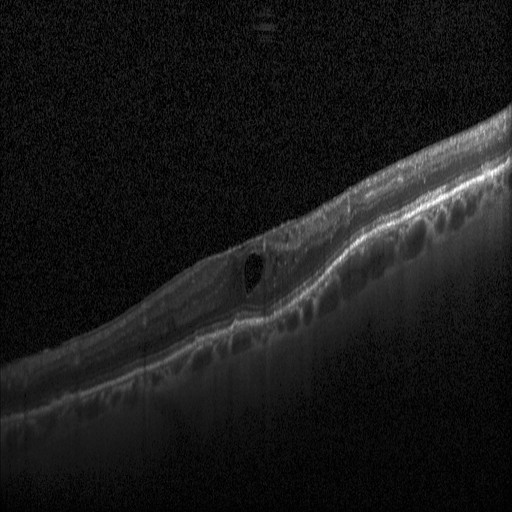

Assessment: DME.